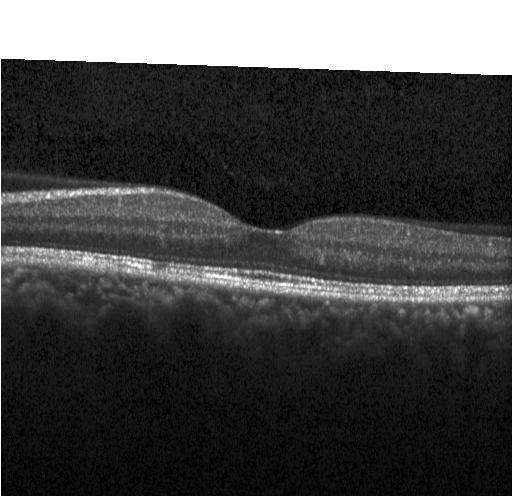 Instrument: Heidelberg Spectralis. Macular scan. SD-OCT. Optical coherence tomography B-scan.
Impression: no choroidal neovascularization, no diabetic macular edema, and no drusen.